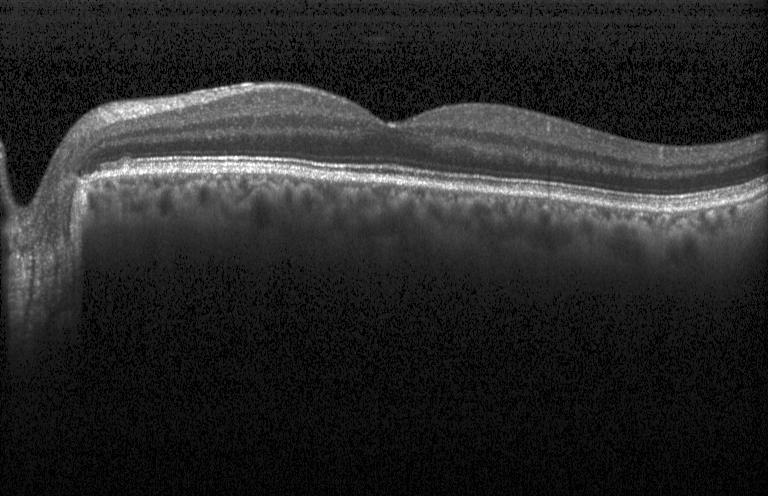 Diagnosis: neither CNV, DME, nor drusen.